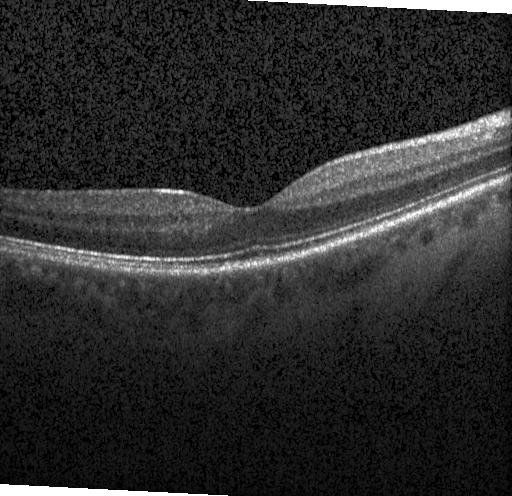
Impression: neither choroidal neovascularization, diabetic macular edema, nor drusen.